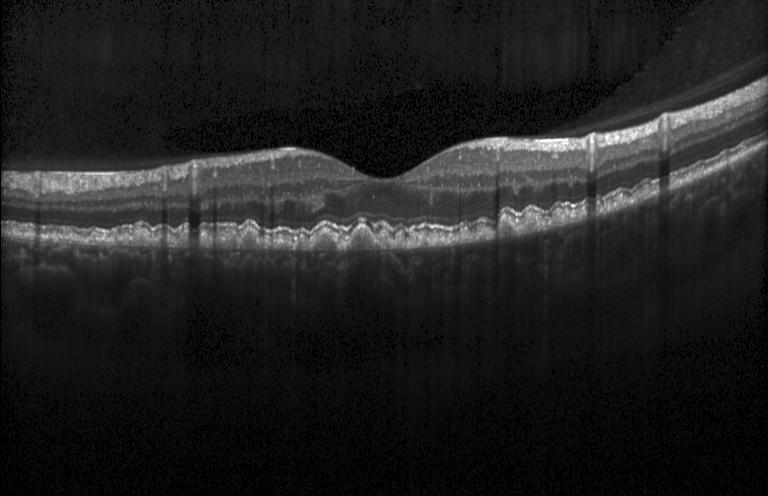 Optical coherence tomography B-scan.
Diagnosis: sub-RPE drusenoid deposits.